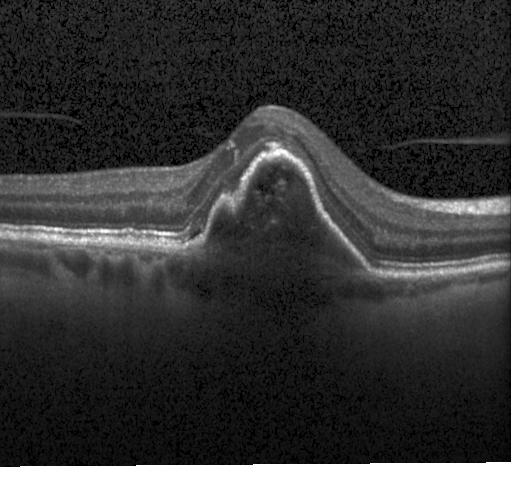
Finding: choroidal neovascularization (CNV).